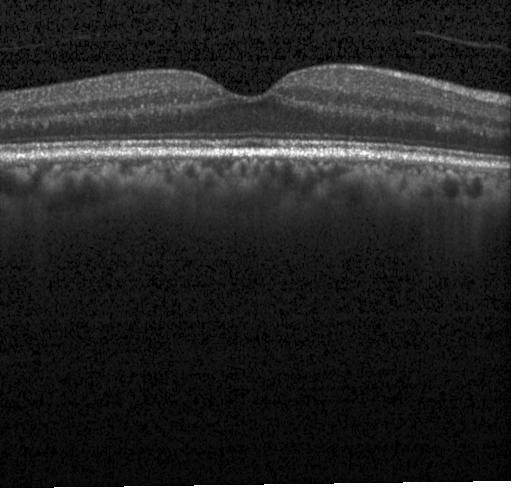

Impression: no evidence of CNV, DME, or drusen.